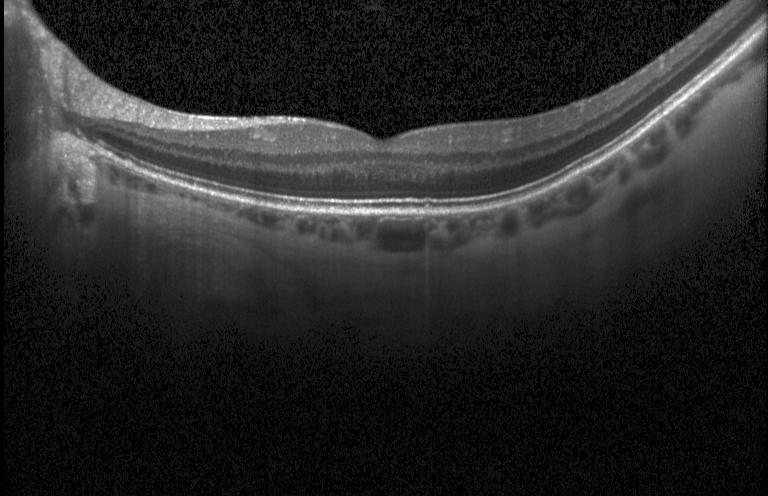 Retinal OCT cross-section.
This B-scan demonstrates multiple drusen.